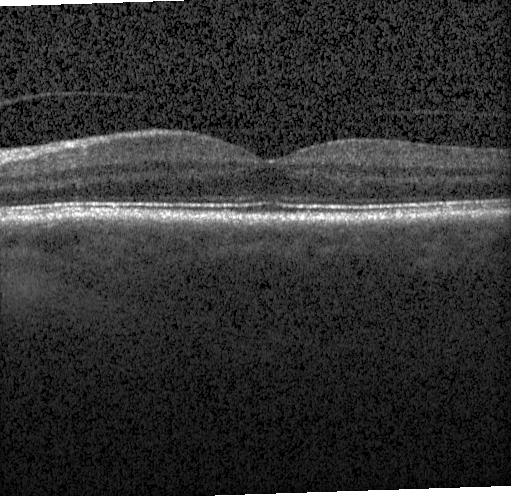 Acquired on a Heidelberg Spectralis, spectral-domain OCT, optical coherence tomography B-scan, through the macula. Finding: neither choroidal neovascularization, diabetic macular edema, nor drusen.